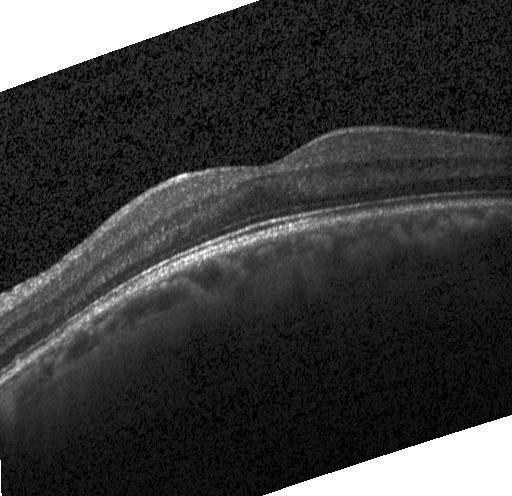

No evidence of choroidal neovascularization, diabetic macular edema, or drusen.